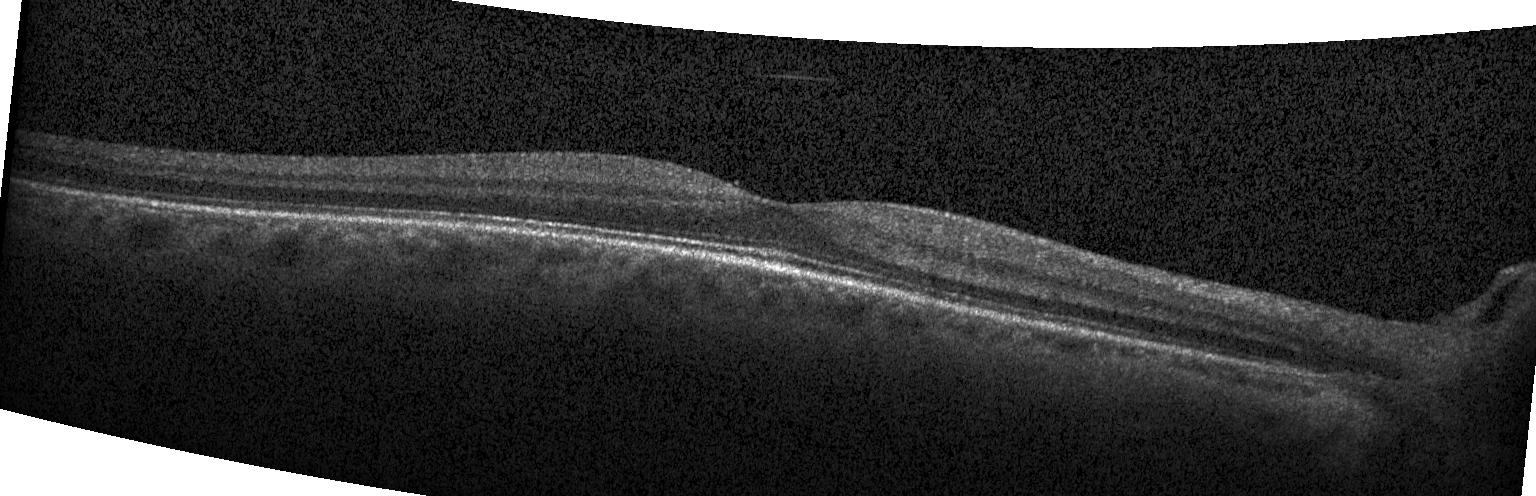
Retinal OCT cross-section showing no CNV, no DME, and no drusen.